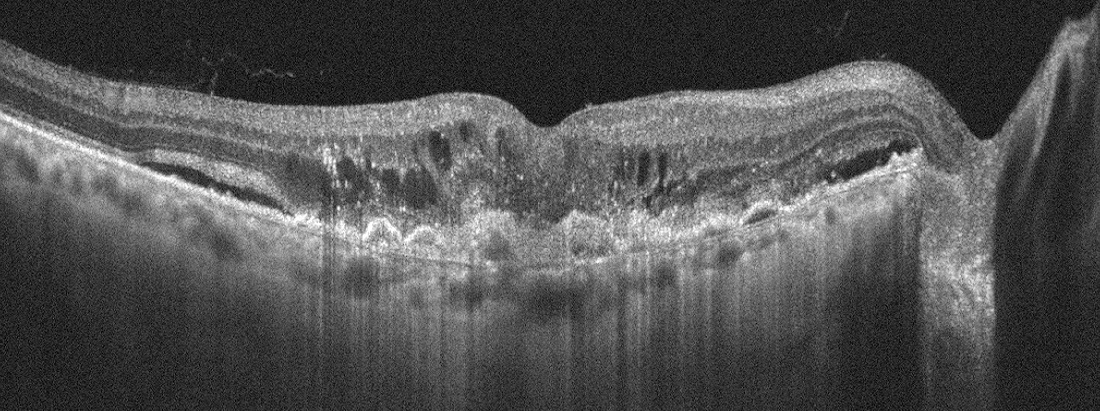 Retinal OCT cross-section · through the macula · instrument: Optovue Avanti RTVue XR
Impression: age-related macular degeneration.